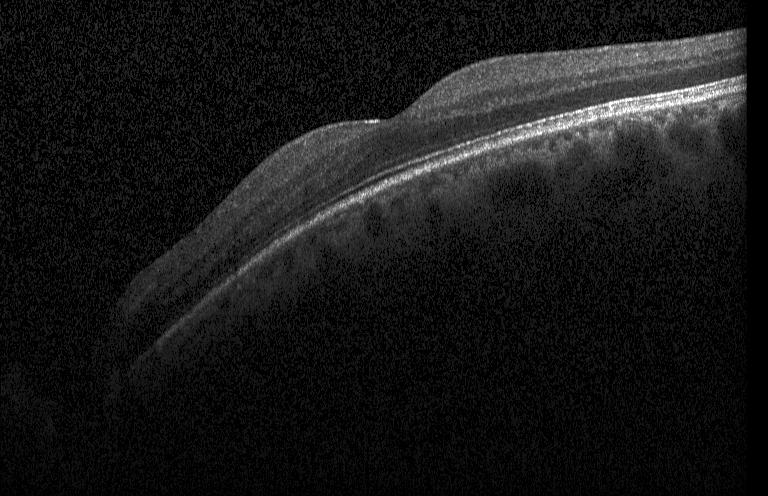
The scan shows neither choroidal neovascularization, diabetic macular edema, nor drusen.